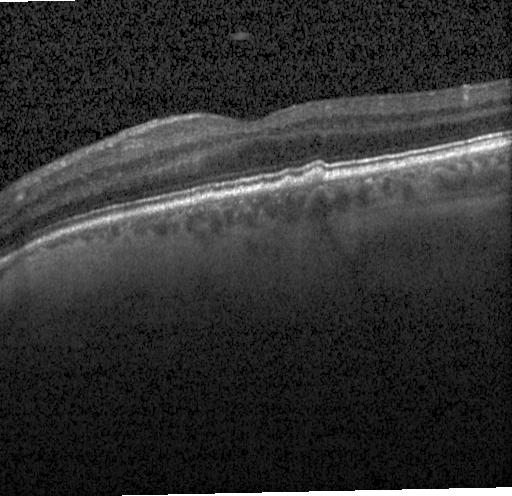 Finding: multiple drusen.